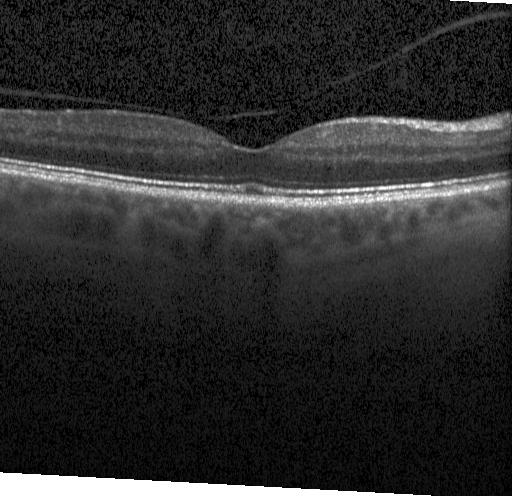 The scan shows no choroidal neovascularization, no diabetic macular edema, and no drusen.